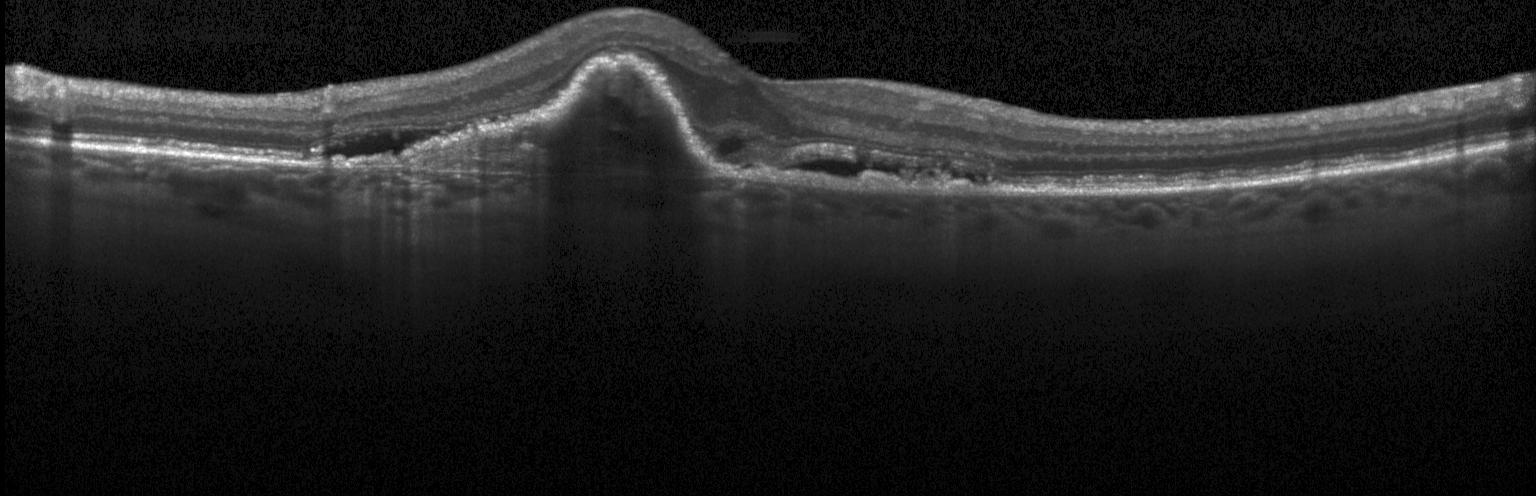

Optical coherence tomography scan. Horizontal scan through the fovea — The scan shows a choroidal neovascular membrane.